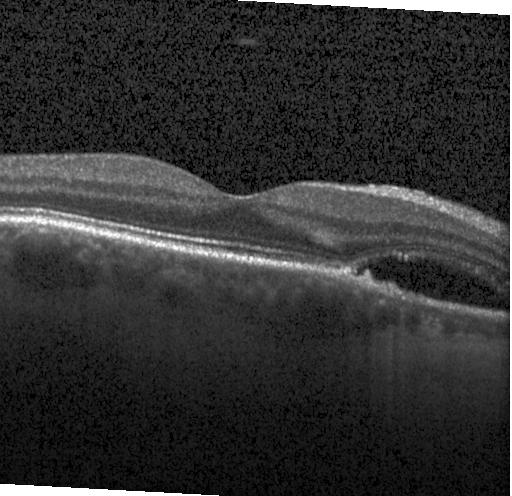
Optical coherence tomography B-scan, acquired on a Heidelberg Spectralis, spectral-domain optical coherence tomography
Dx: a choroidal neovascular membrane.